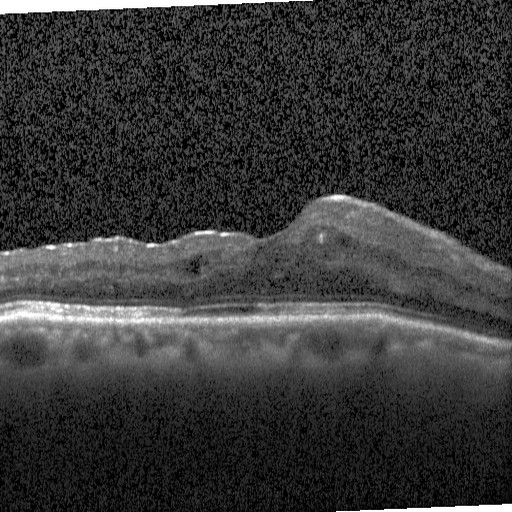

Retinal OCT cross-section, SD-OCT
Impression: diabetic macular edema (DME).